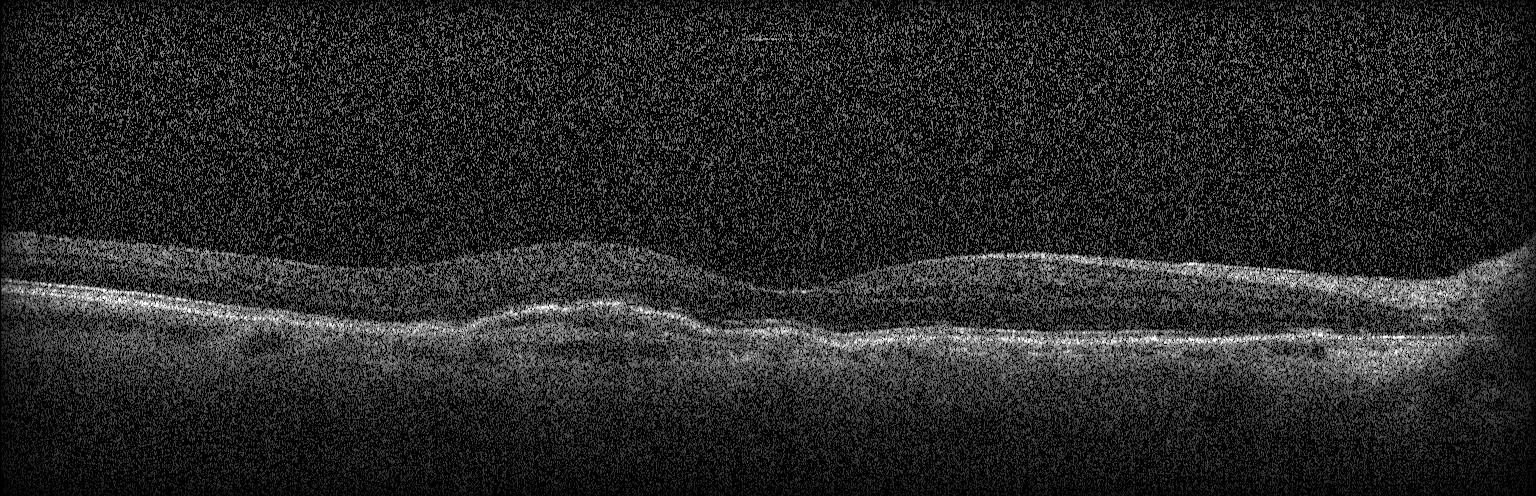
Finding: choroidal neovascularization.